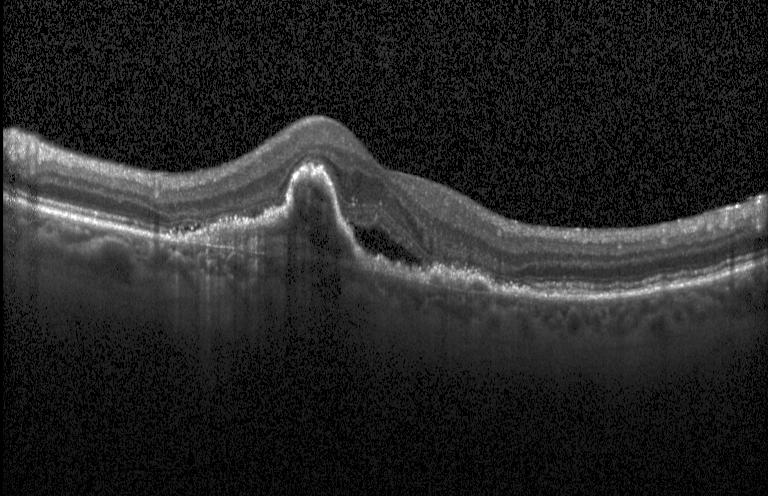

Retinal OCT B-scan. Fovea-centered. Acquired on a Heidelberg Spectralis. Dx: CNV.